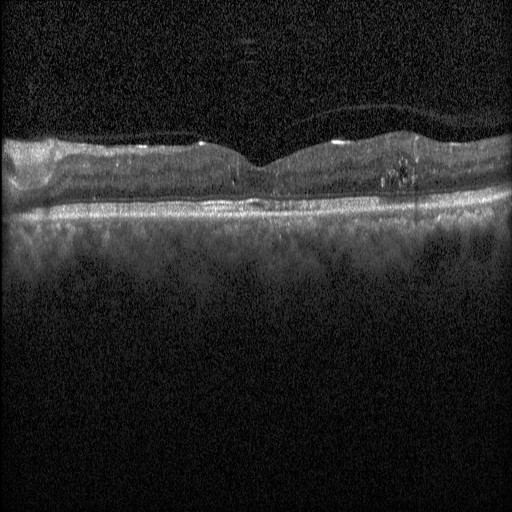 Finding: diabetic macular edema (DME).